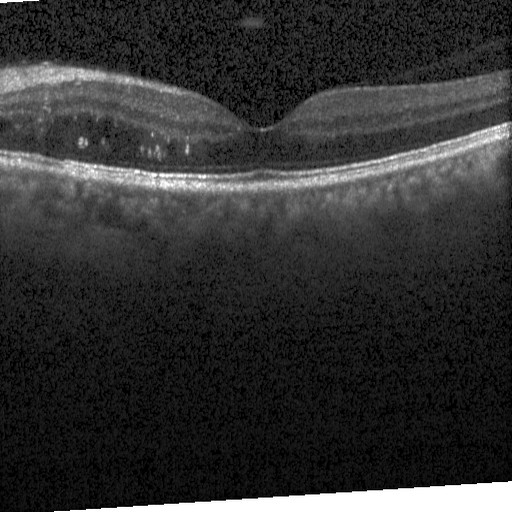 Diagnosis: diabetic macular edema.